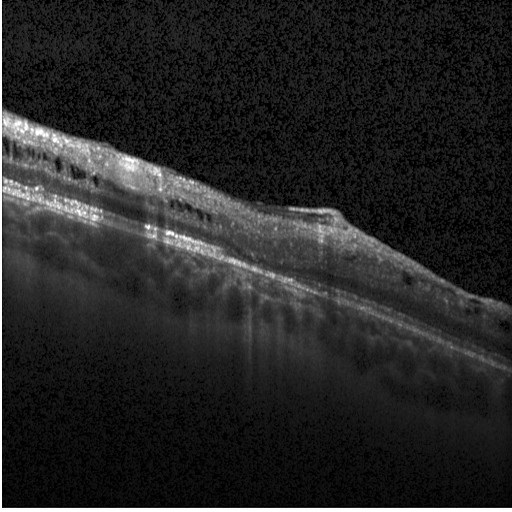

Macular OCT: DME.